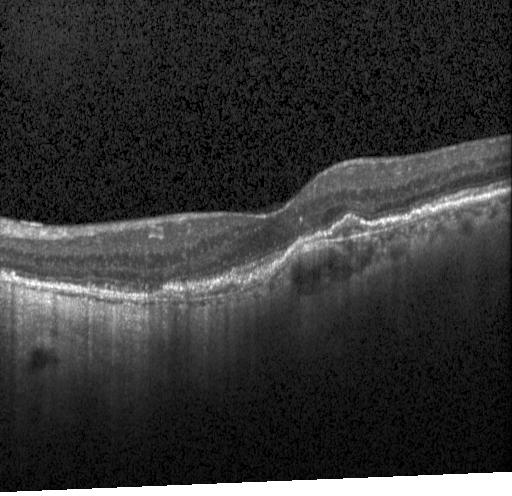
Finding: choroidal neovascularization.